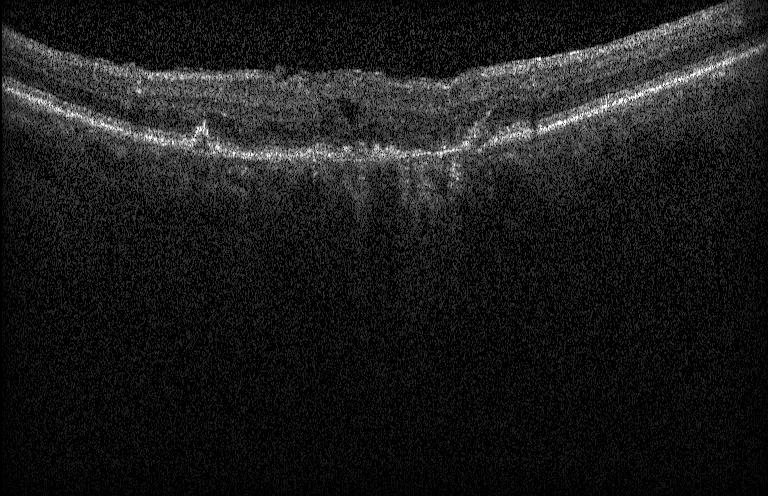 Optical coherence tomography scan. Diagnosis: choroidal neovascularization (CNV).